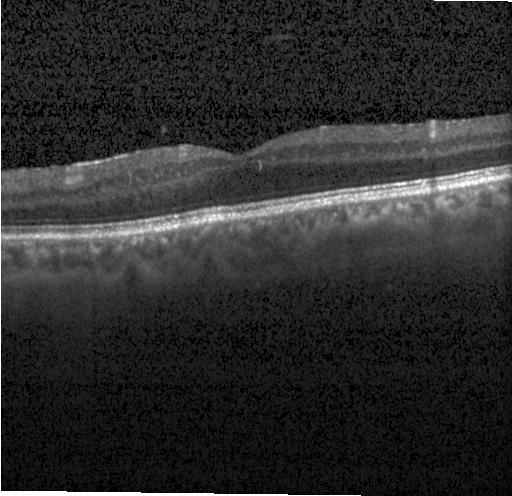

Diagnosis: neither choroidal neovascularization, diabetic macular edema, nor drusen.